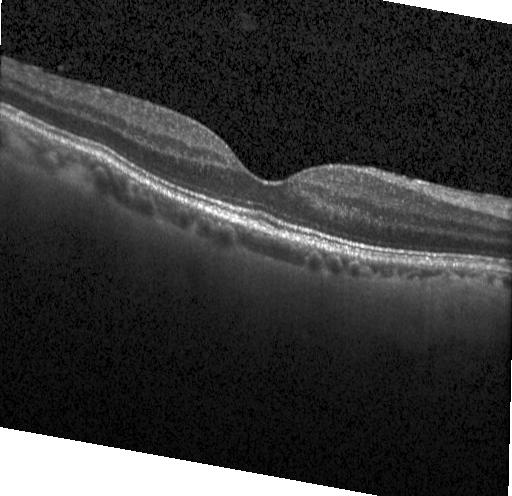

Retinal OCT cross-section. Spectral-domain OCT. Horizontal scan through the fovea
Assessment: neither CNV, DME, nor drusen.